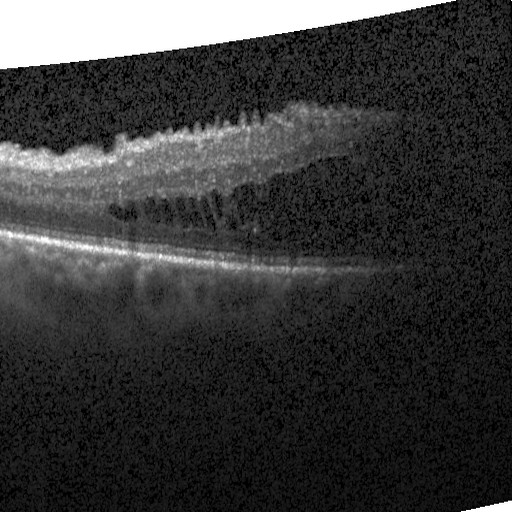 OCT B-scan showing DME.